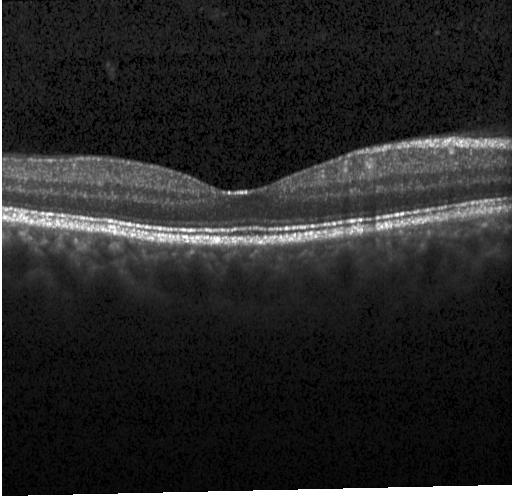

Retinal OCT cross-section, through the macula, Heidelberg Spectralis, spectral-domain optical coherence tomography.
This B-scan demonstrates neither CNV, DME, nor drusen.